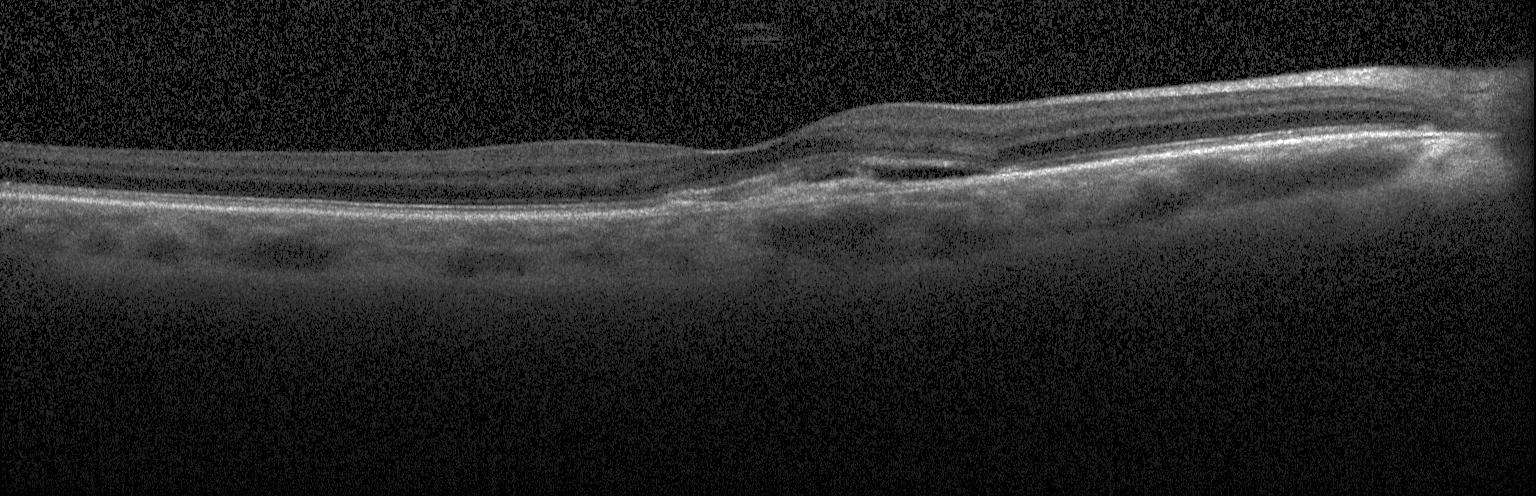
Macular OCT demonstrating a choroidal neovascular membrane.